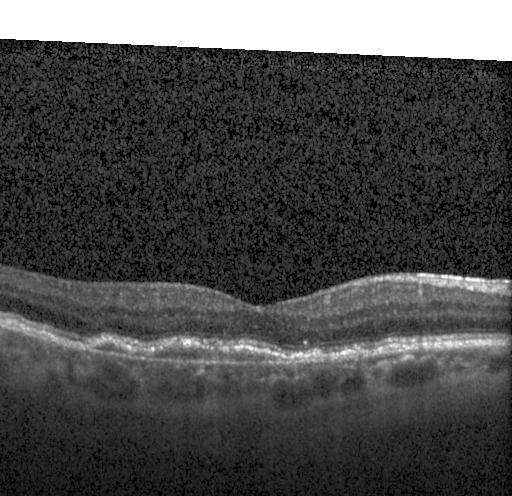
Macular scan. OCT line scan — The scan shows choroidal neovascularization (CNV).